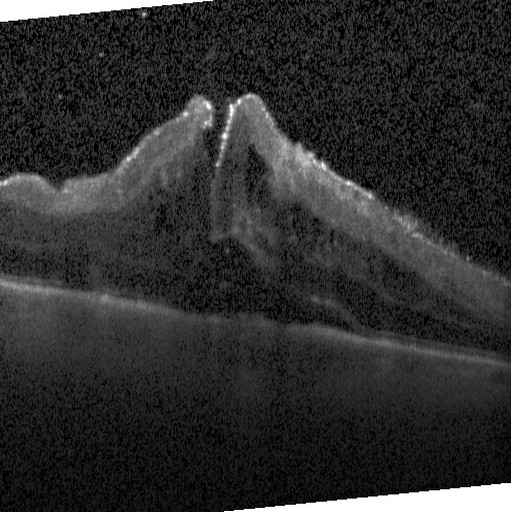
Spectral-domain OCT. Acquired on a Heidelberg Spectralis. Retinal OCT B-scan. Through the macula. Impression: diabetic macular edema (DME).